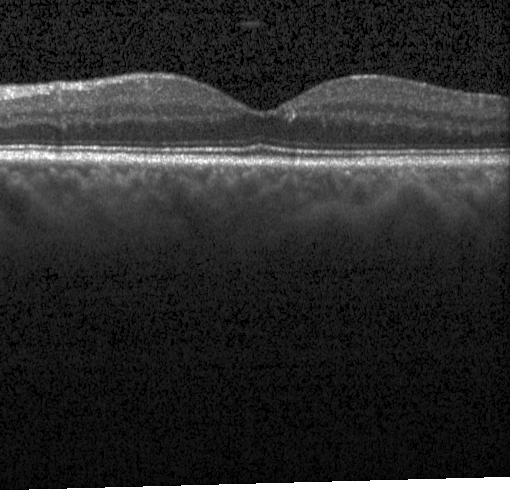 Dx: no choroidal neovascularization, diabetic macular edema, or drusen.